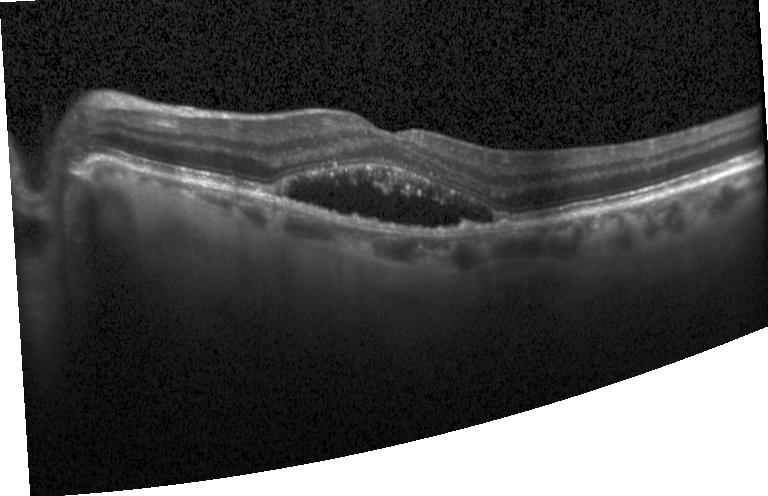
Dx: a choroidal neovascular membrane.